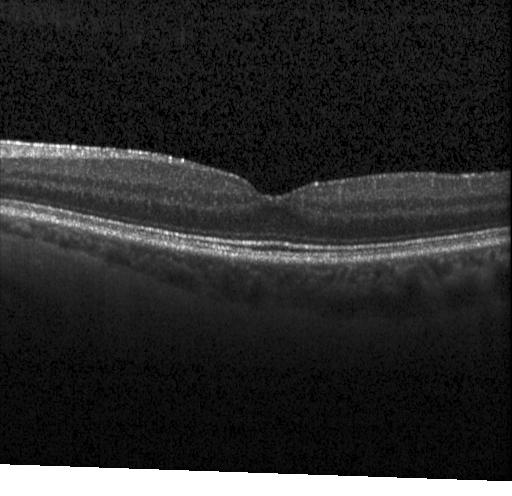 Retinal OCT cross-section; macular scan; spectral-domain optical coherence tomography
Impression: no CNV, DME, or drusen.